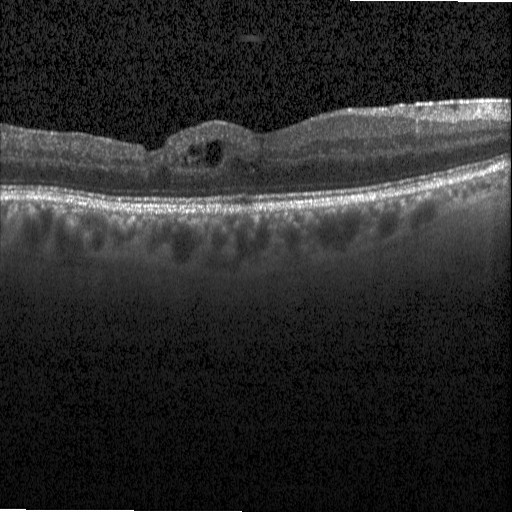

Macular OCT demonstrating DME.